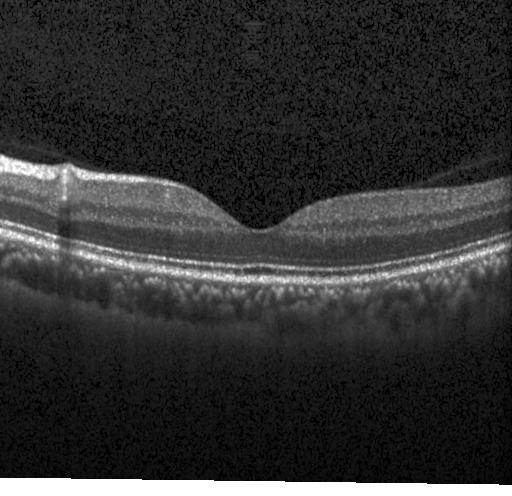

No evidence of choroidal neovascularization, diabetic macular edema, or drusen.